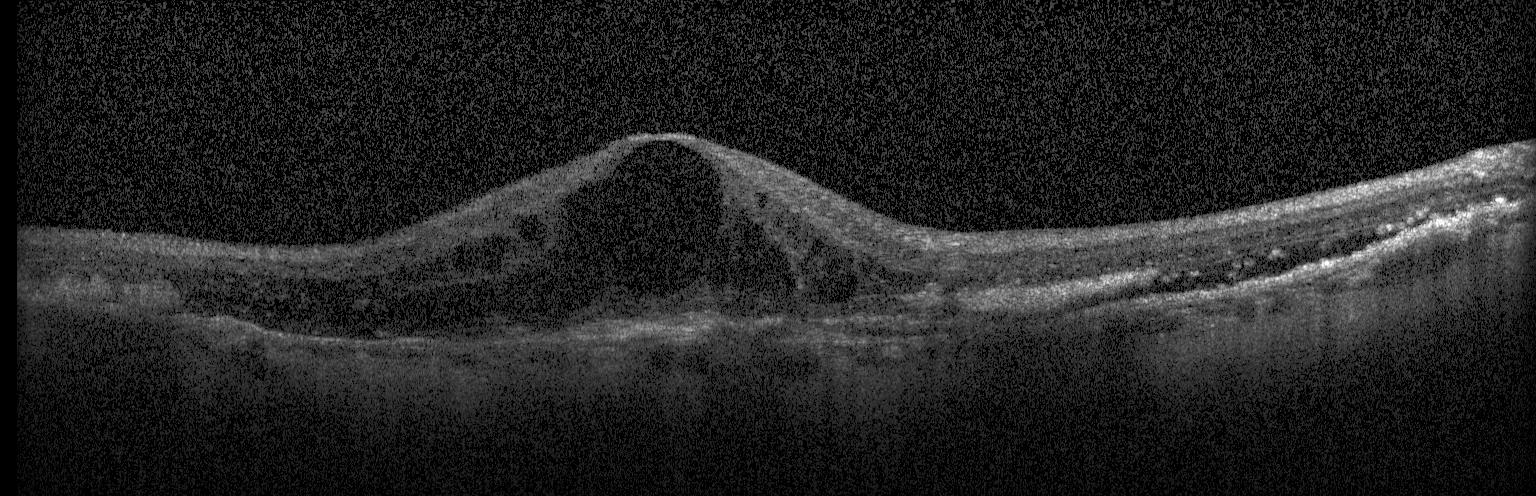
Spectral-domain OCT; centered on the fovea; acquired on a Heidelberg Spectralis; retinal OCT B-scan — Assessment: choroidal neovascularization (CNV).